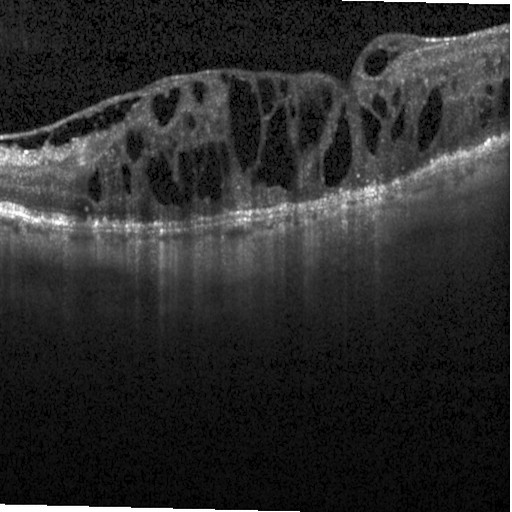
Retinal OCT cross-section, instrument: Heidelberg Spectralis
OCT finding: diabetic macular edema.